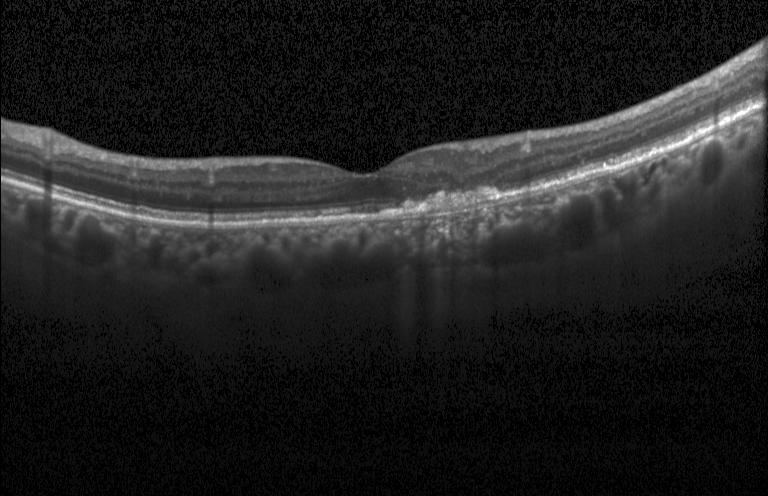 OCT line scan; SD-OCT. Diagnosis: a choroidal neovascular membrane.